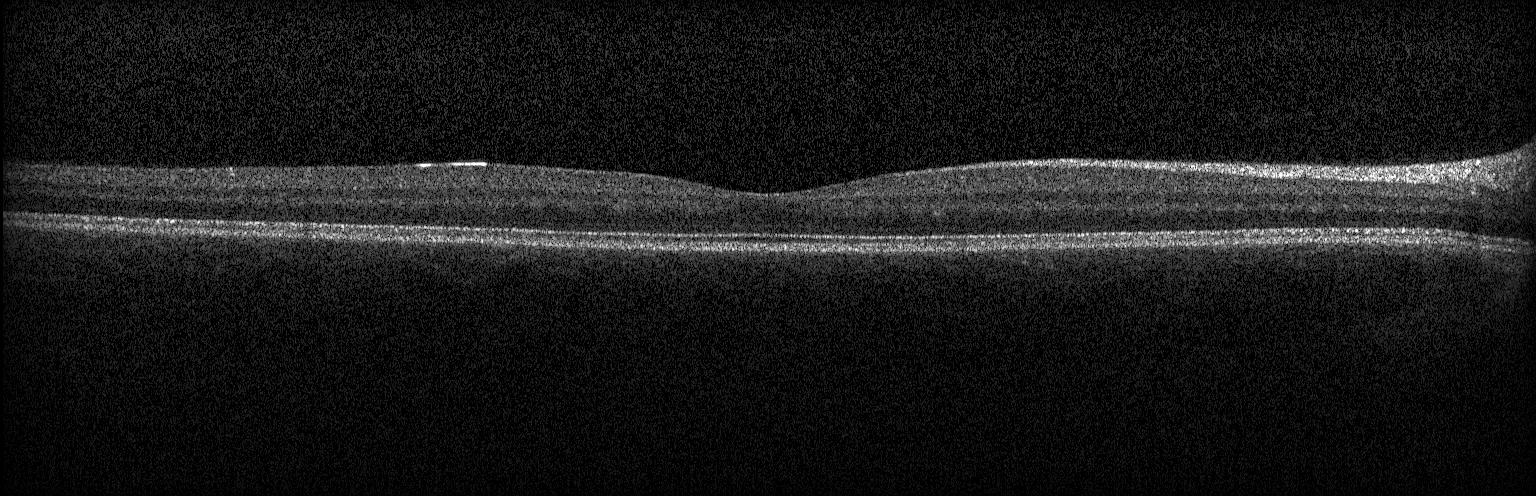
Optical coherence tomography B-scan.
This B-scan demonstrates no evidence of CNV, DME, or drusen.